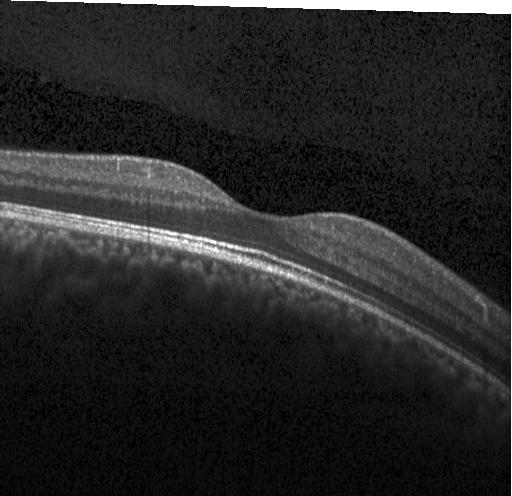

Retinal OCT B-scan; spectral-domain optical coherence tomography. Macular OCT: no choroidal neovascularization, diabetic macular edema, or drusen.